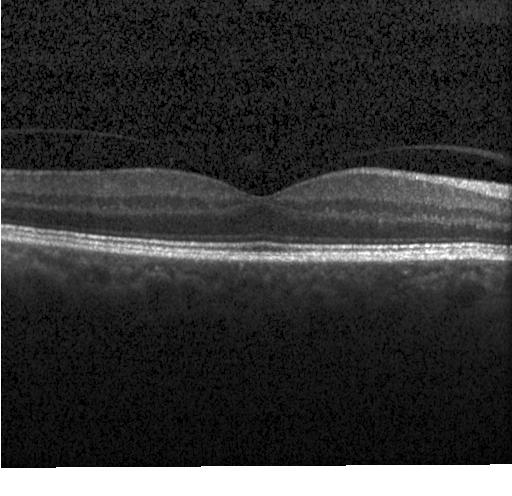

Horizontal scan through the fovea. Heidelberg Spectralis OCT system. Spectral-domain OCT. Optical coherence tomography B-scan. Diagnosis: neither CNV, DME, nor drusen.